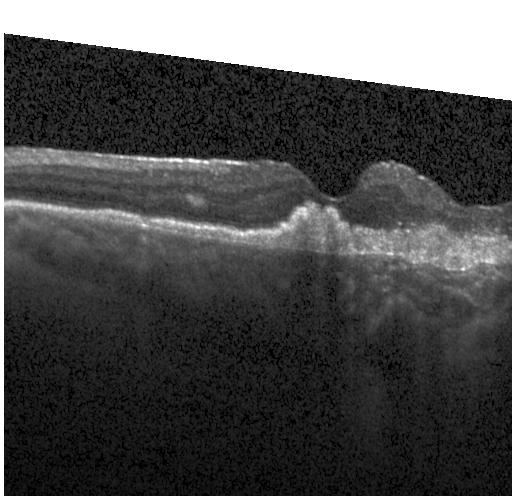 OCT finding: CNV.